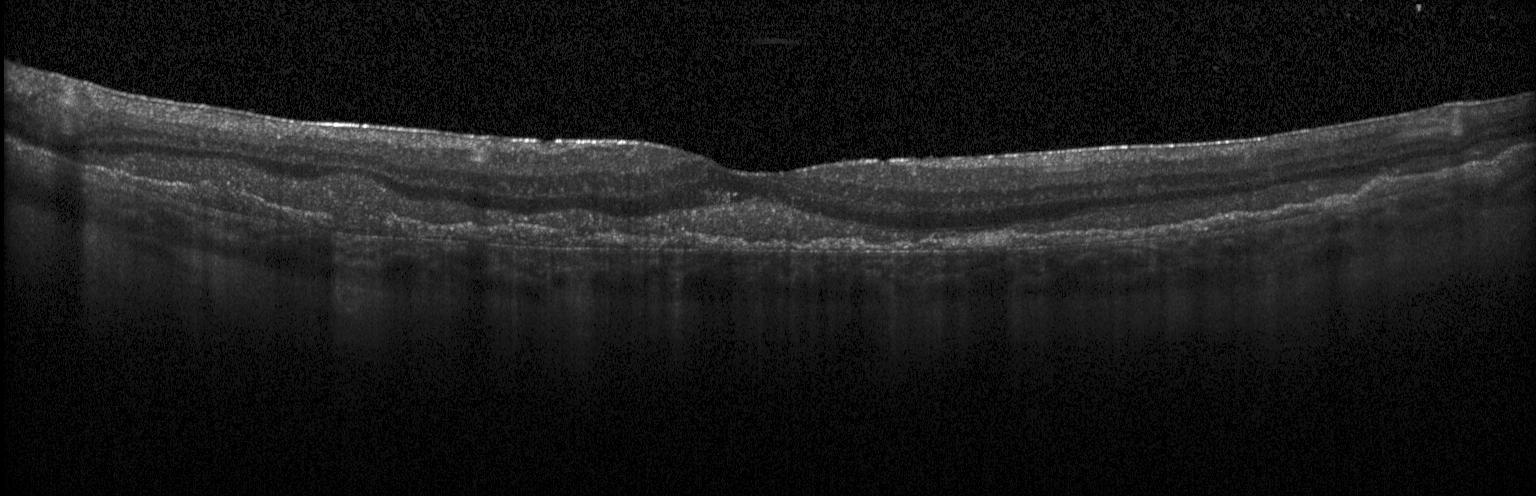

OCT line scan
Assessment: a choroidal neovascular membrane.